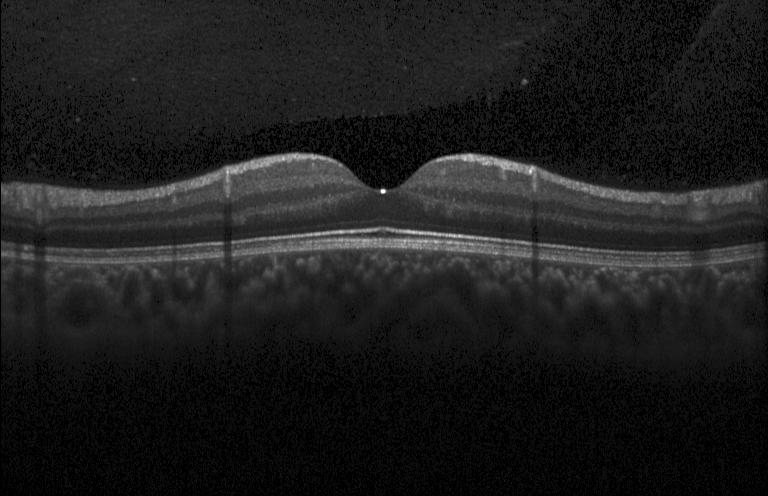
OCT B-scan; acquired on a Heidelberg Spectralis; SD-OCT; macular scan
The scan shows no CNV, no DME, and no drusen.